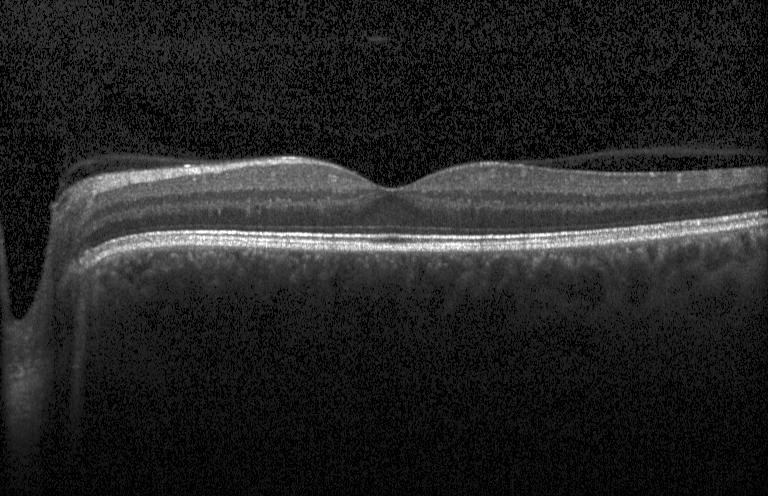

Retinal OCT cross-section showing neither CNV, DME, nor drusen.